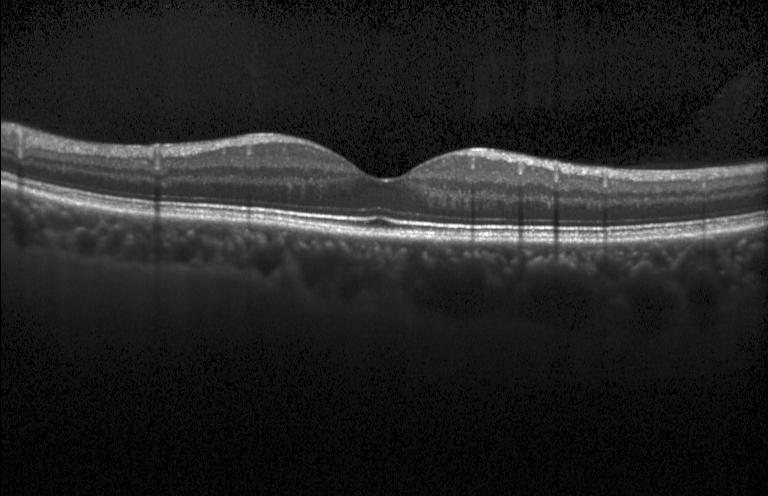 Neither CNV, DME, nor drusen.